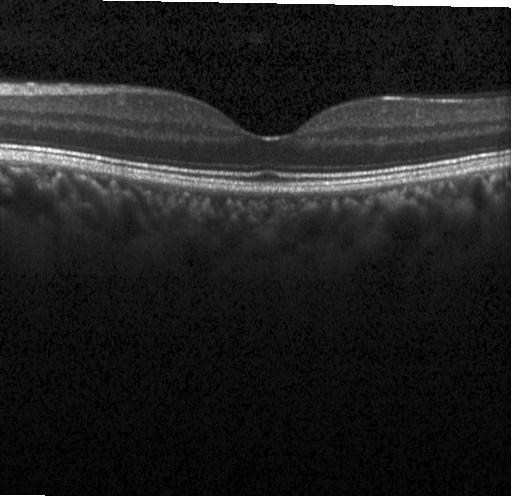

Retinal OCT B-scan. Impression: no choroidal neovascularization, diabetic macular edema, or drusen.